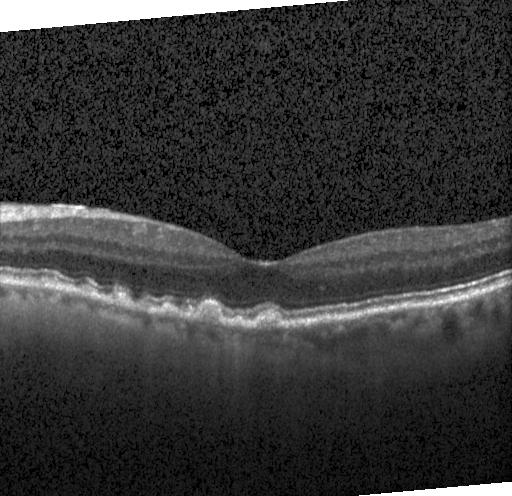
Diagnosis: sub-RPE drusenoid deposits.